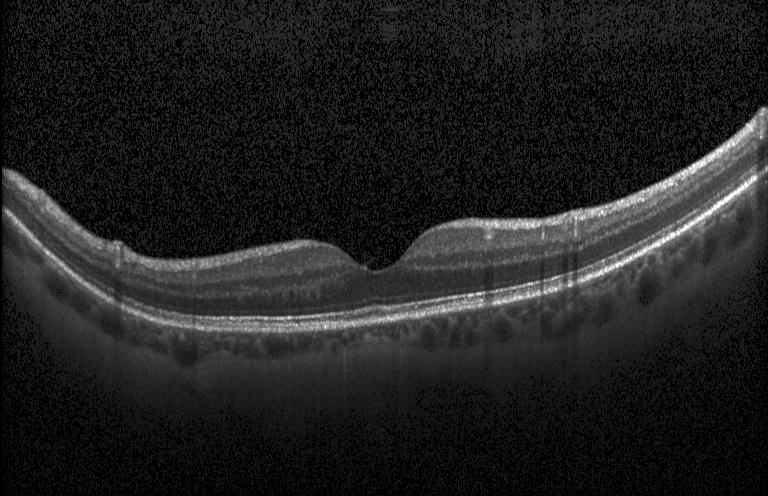
Macular scan, OCT line scan.
Finding: no choroidal neovascularization, diabetic macular edema, or drusen.